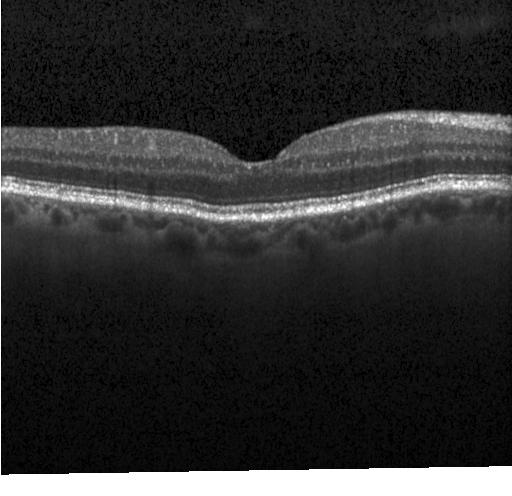 Horizontal scan through the fovea · retinal OCT cross-section · acquired on a Heidelberg Spectralis.
Dx: no evidence of choroidal neovascularization, diabetic macular edema, or drusen.